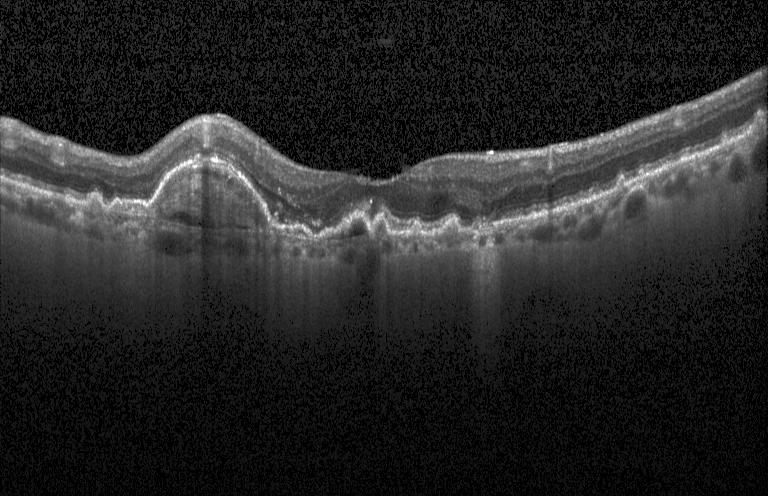

OCT B-scan — Finding: choroidal neovascularization (CNV).